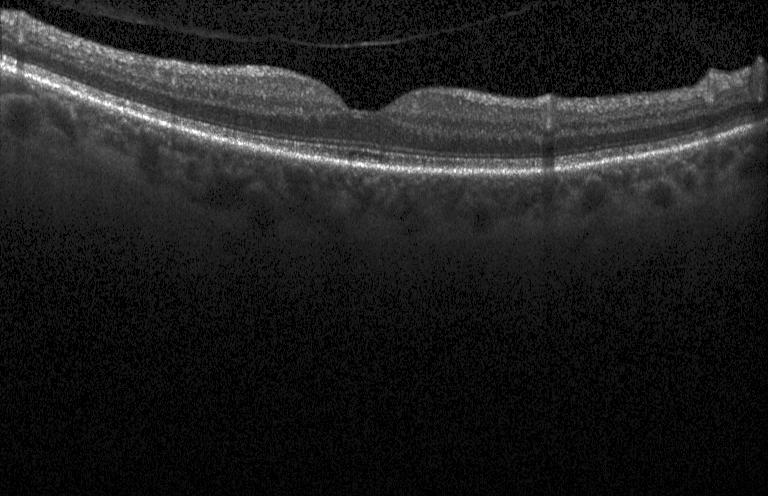

Heidelberg Spectralis OCT system. Through the macula. SD-OCT. Retinal OCT cross-section
Diagnosis: no evidence of choroidal neovascularization, diabetic macular edema, or drusen.